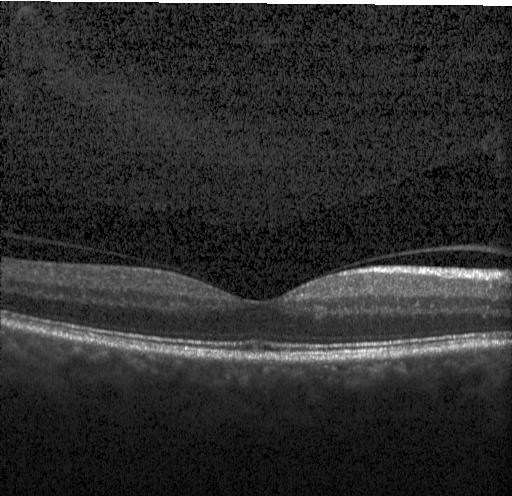

Dx: no choroidal neovascularization, diabetic macular edema, or drusen.